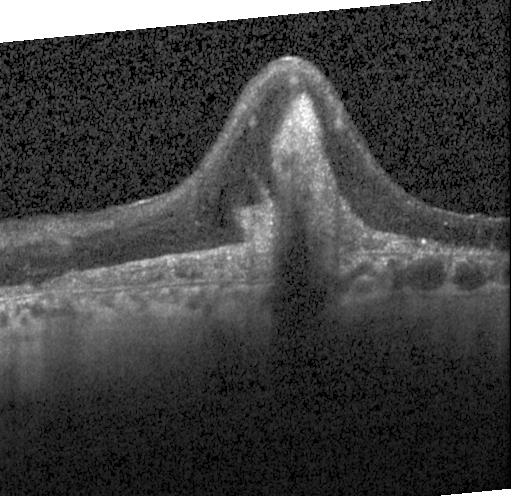 Fovea-centered, SD-OCT, OCT line scan
The scan shows choroidal neovascularization (CNV).